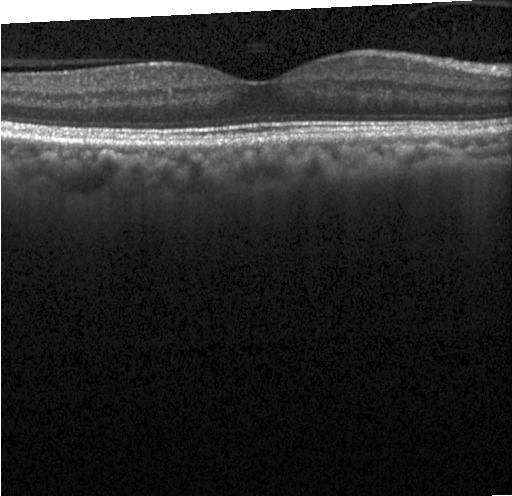
Heidelberg Spectralis, optical coherence tomography B-scan, spectral-domain optical coherence tomography.
The scan shows no CNV, DME, or drusen.